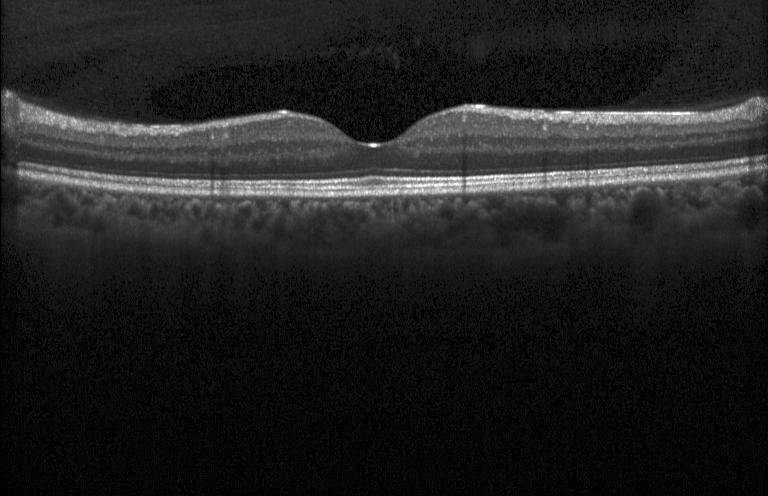
Through the macula, instrument: Heidelberg Spectralis, spectral-domain optical coherence tomography, optical coherence tomography scan — Diagnosis: no evidence of choroidal neovascularization, diabetic macular edema, or drusen.